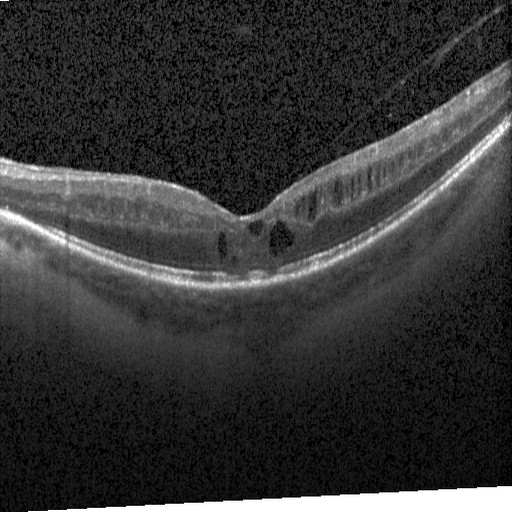

Heidelberg Spectralis OCT system, optical coherence tomography B-scan, through the macula.
Dx: DME.